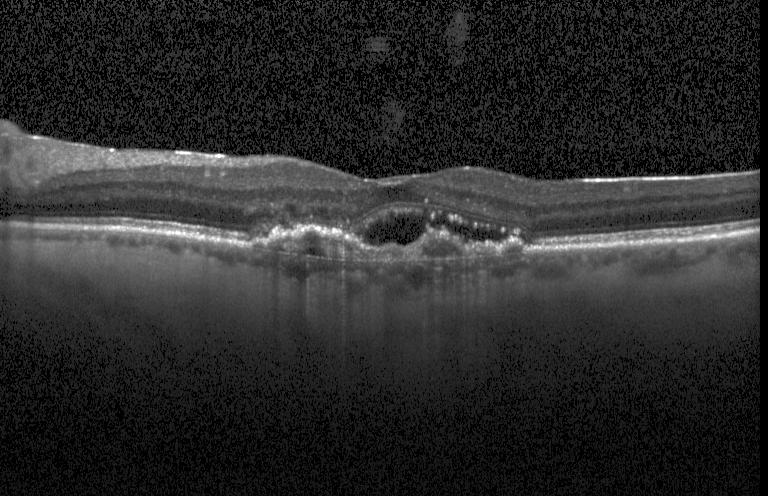
Acquired on a Heidelberg Spectralis · OCT line scan
Finding: a choroidal neovascular membrane.